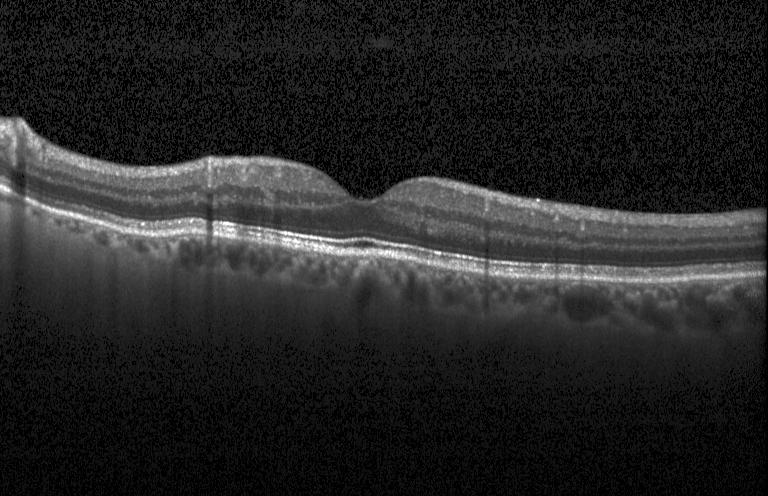

Through the macula, OCT line scan, SD-OCT
OCT finding: no CNV, DME, or drusen.